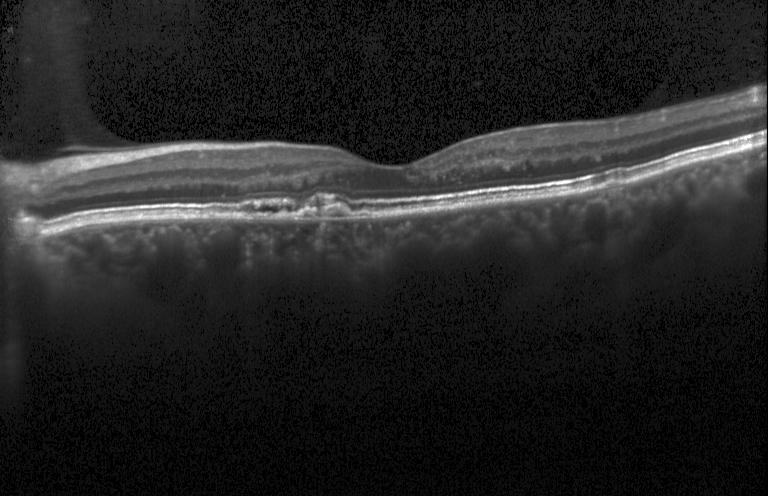 Macular OCT: choroidal neovascularization (CNV).